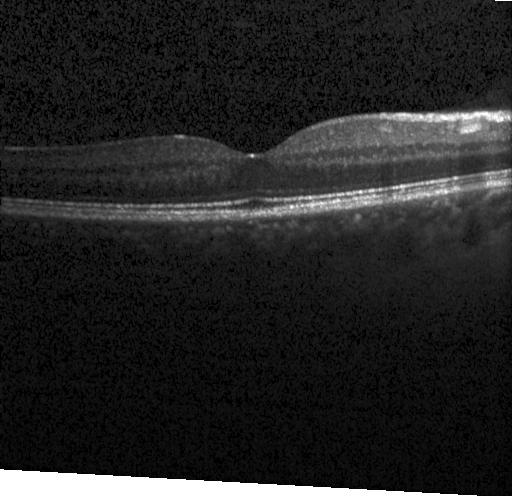

Diagnosis: neither CNV, DME, nor drusen.